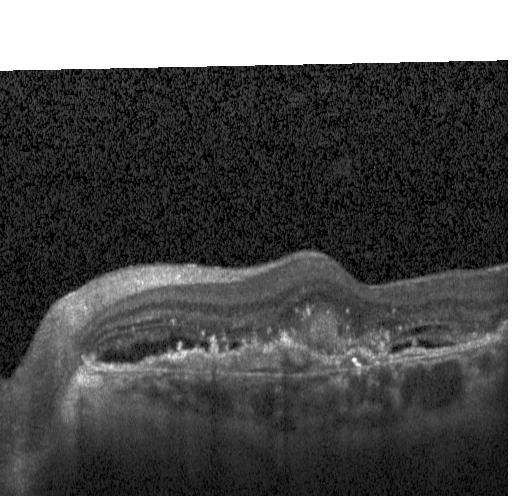 Finding: a choroidal neovascular membrane.